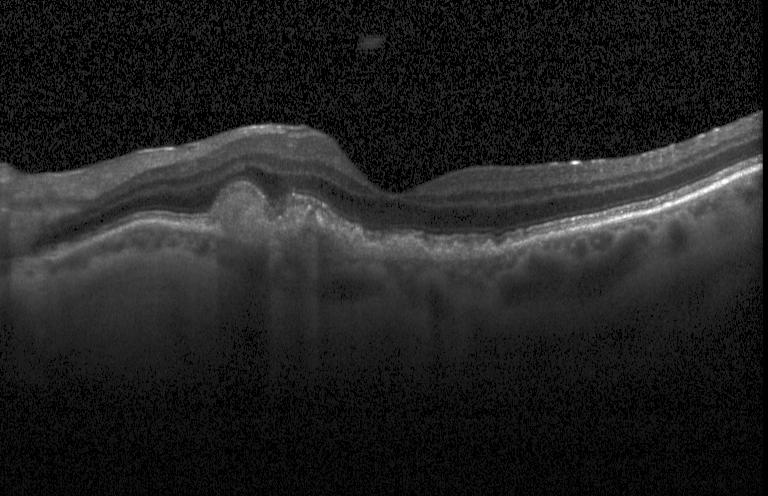

Macular OCT: choroidal neovascularization.